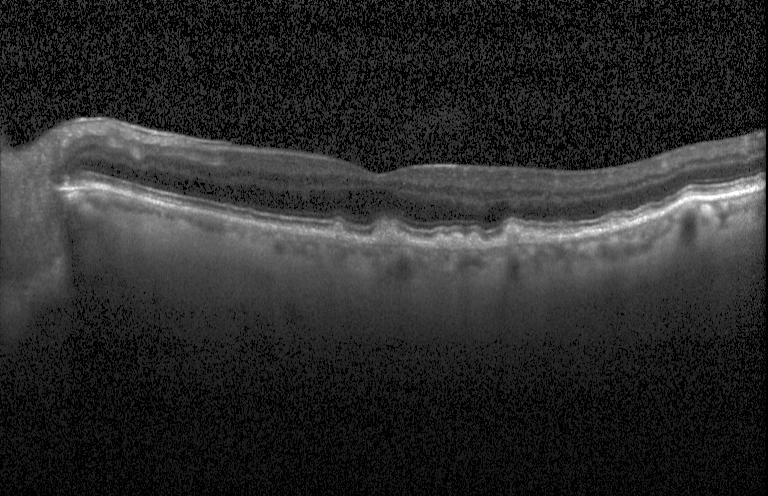
Spectral-domain OCT, Heidelberg Spectralis OCT system, OCT line scan. Drusen.